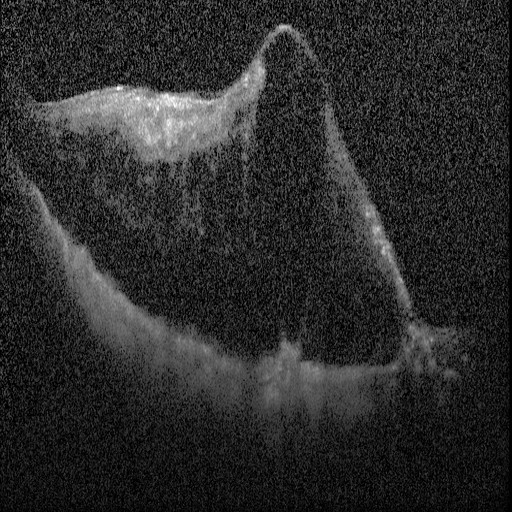 Retinal OCT cross-section
This B-scan demonstrates DME.